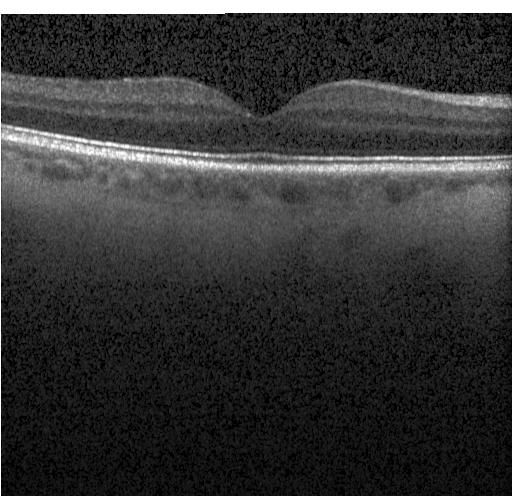 Retinal OCT cross-section.
Diagnosis: neither choroidal neovascularization, diabetic macular edema, nor drusen.